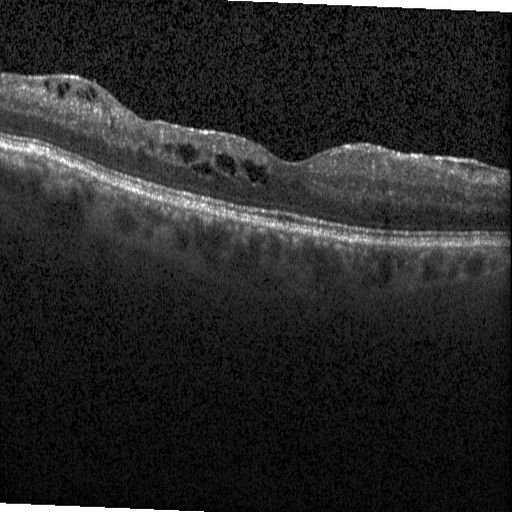
Retinal OCT B-scan. Impression: diabetic macular edema (DME).